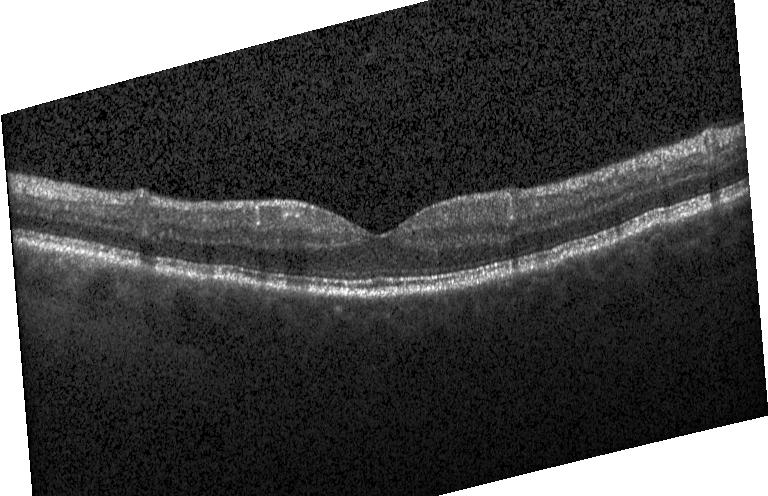

Optical coherence tomography B-scan.
This B-scan demonstrates no choroidal neovascularization, no diabetic macular edema, and no drusen.